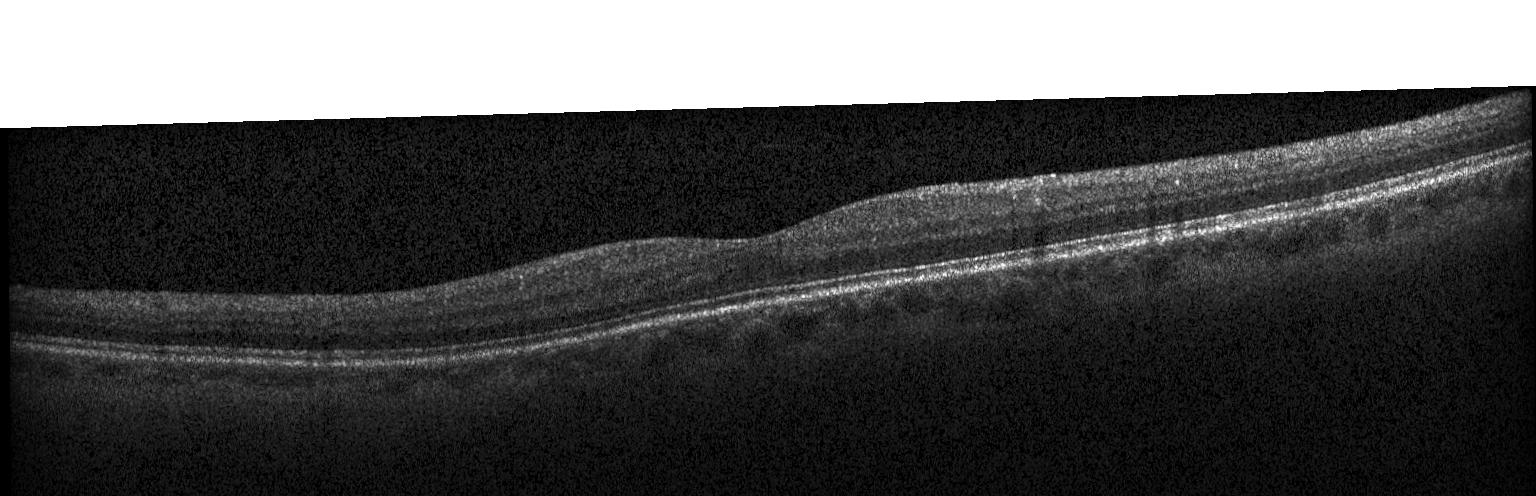
Centered on the fovea · OCT B-scan · SD-OCT.
Dx: no evidence of choroidal neovascularization, diabetic macular edema, or drusen.